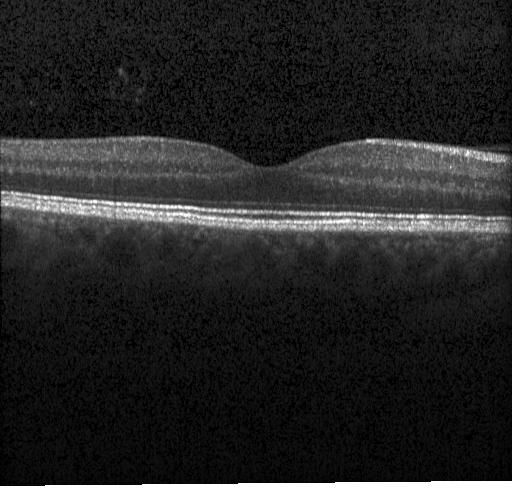

Optical coherence tomography scan, through the macula. Impression: no evidence of choroidal neovascularization, diabetic macular edema, or drusen.